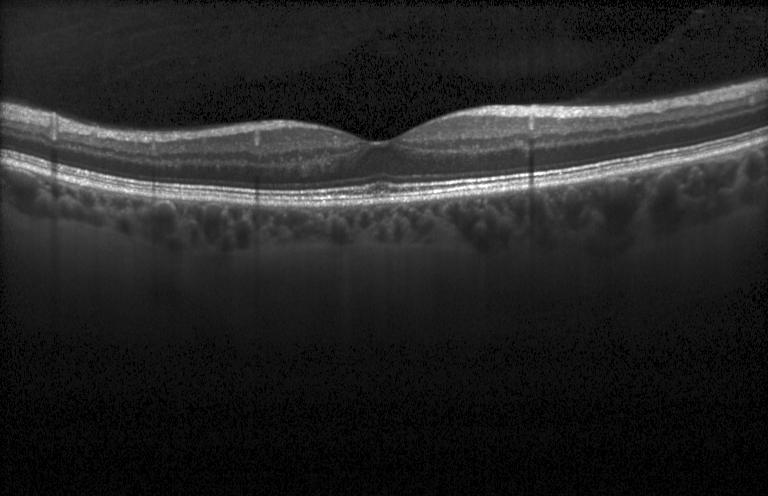
SD-OCT; retinal OCT cross-section; acquired on a Heidelberg Spectralis — Finding: neither CNV, DME, nor drusen.